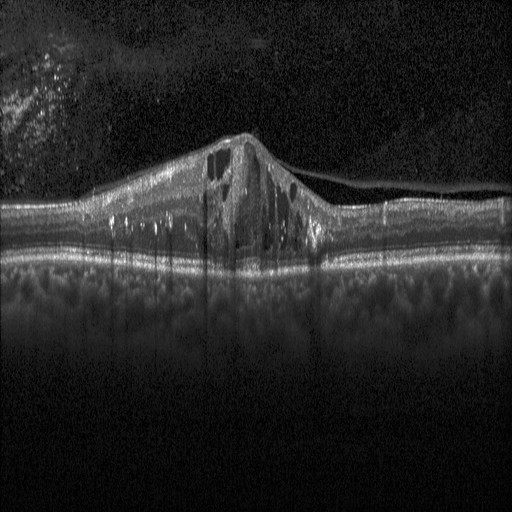
Macular OCT: DME.